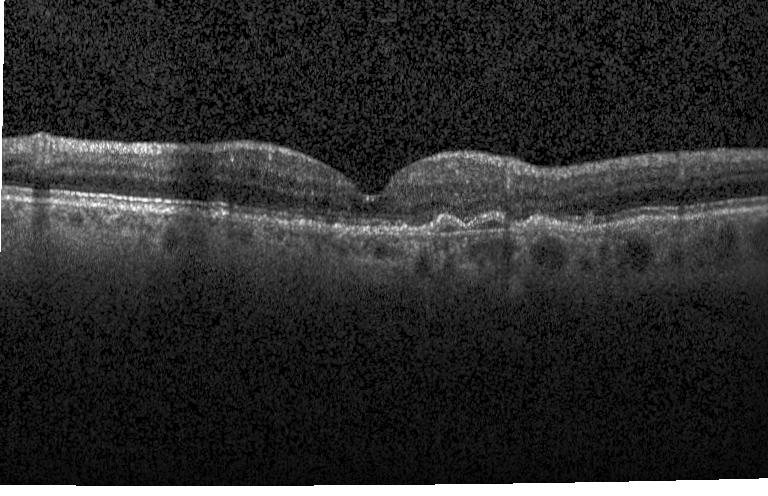
Retinal OCT cross-section showing a choroidal neovascular membrane.